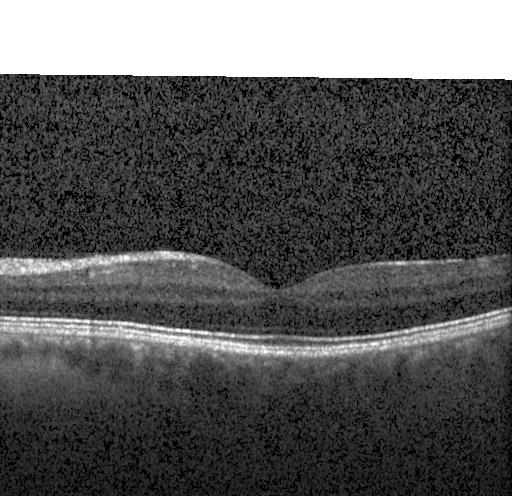

Retinal OCT cross-section · spectral-domain OCT · macular scan — OCT finding: neither choroidal neovascularization, diabetic macular edema, nor drusen.